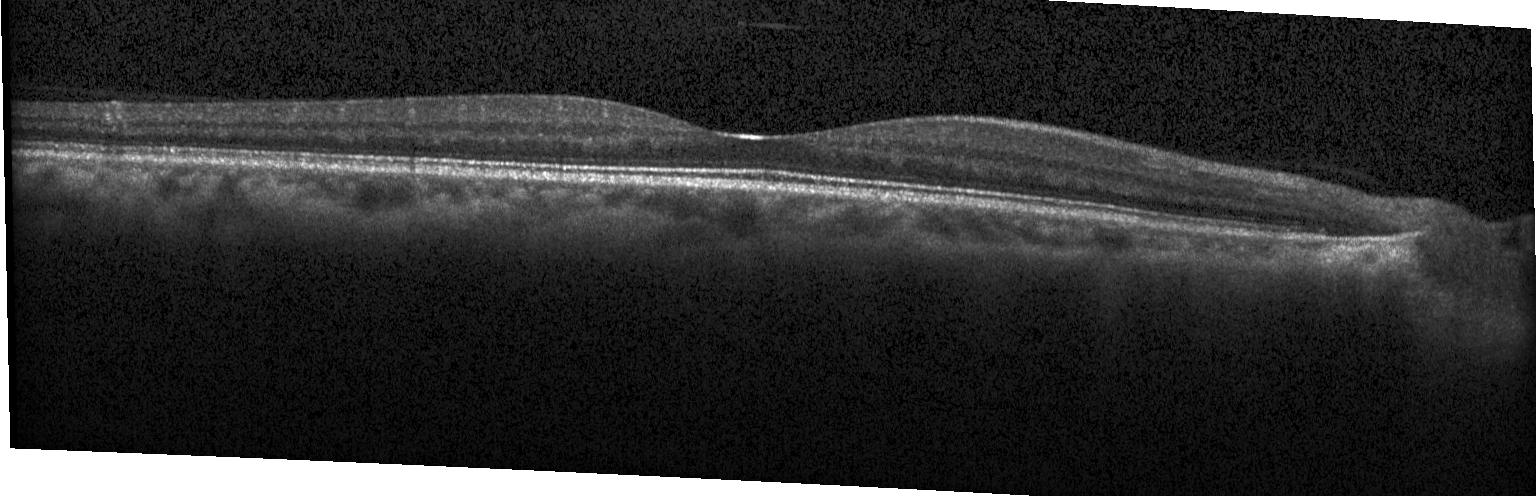
Spectral-domain OCT · retinal OCT cross-section — The scan shows neither choroidal neovascularization, diabetic macular edema, nor drusen.